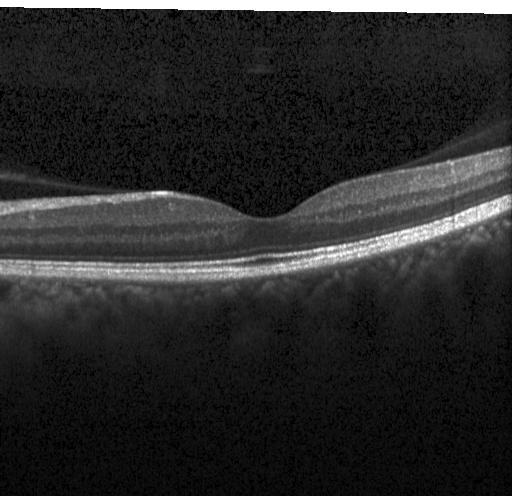

Assessment: no choroidal neovascularization, no diabetic macular edema, and no drusen.